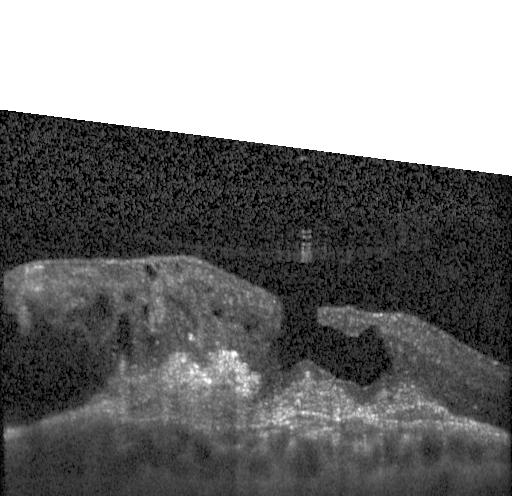
Spectral-domain optical coherence tomography; OCT line scan; horizontal scan through the fovea. Diagnosis: a choroidal neovascular membrane.